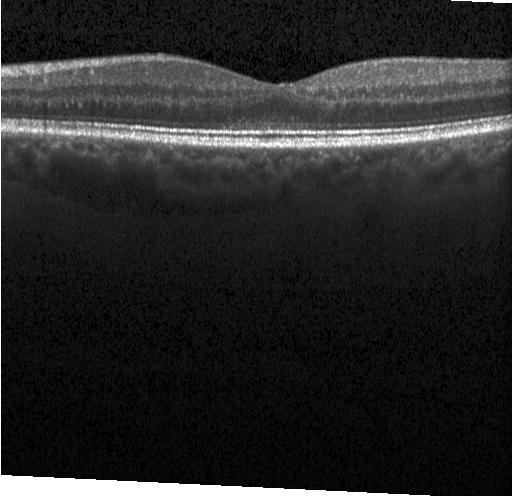

Dx: no evidence of CNV, DME, or drusen.